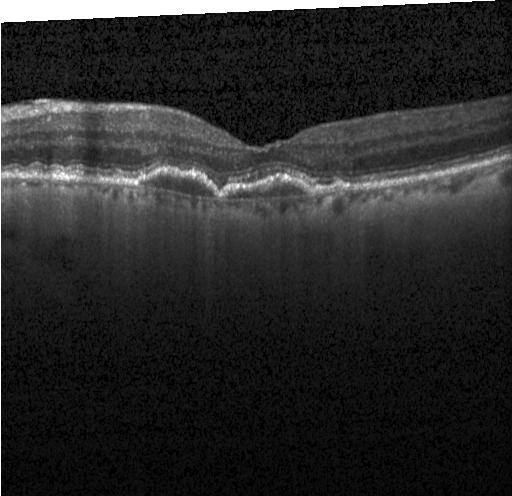
OCT line scan. Acquired on a Heidelberg Spectralis. Fovea-centered — Diagnosis: CNV.